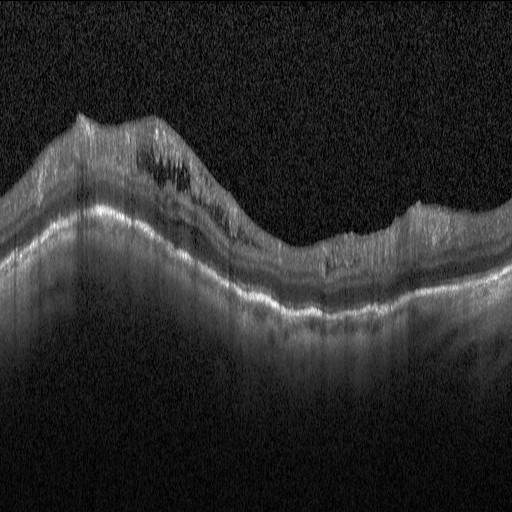 Spectral-domain OCT B-scan: diabetic macular edema (DME).